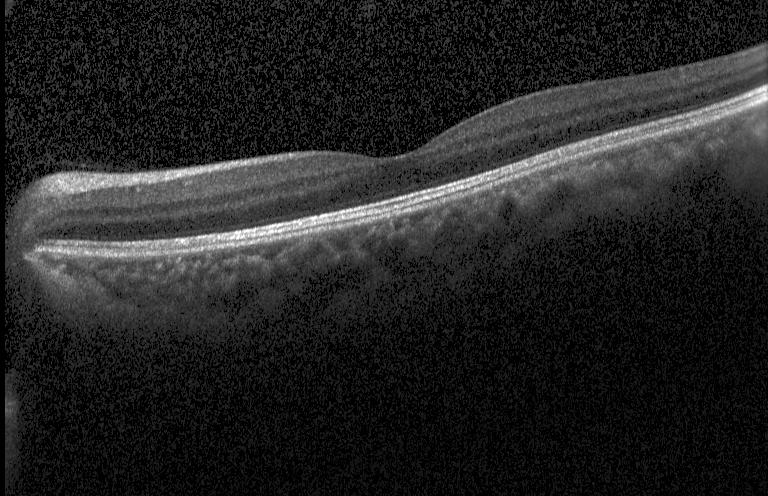
Retinal OCT B-scan — Diagnosis: neither choroidal neovascularization, diabetic macular edema, nor drusen.